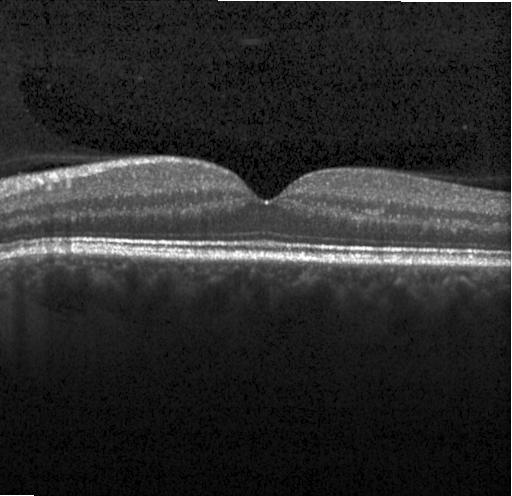 SD-OCT; centered on the fovea; Heidelberg Spectralis OCT system; OCT B-scan. Neither choroidal neovascularization, diabetic macular edema, nor drusen.